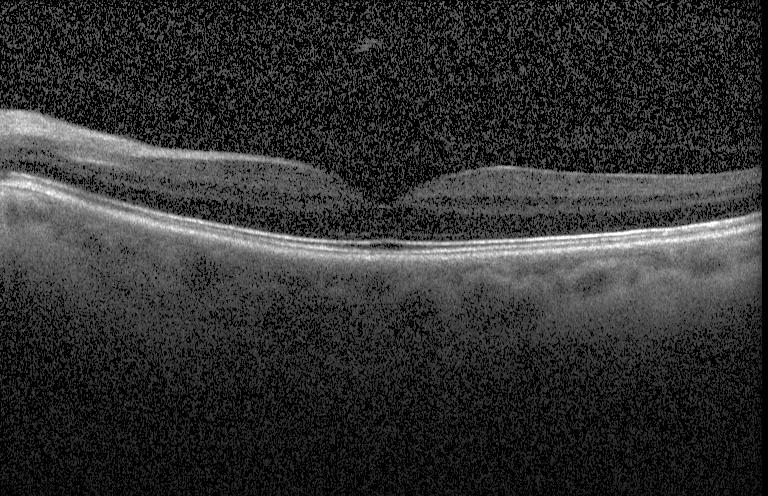

This B-scan demonstrates no choroidal neovascularization, diabetic macular edema, or drusen.